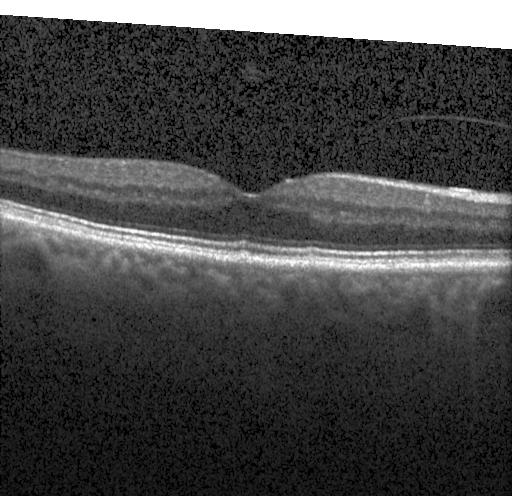 OCT finding: no choroidal neovascularization, diabetic macular edema, or drusen.